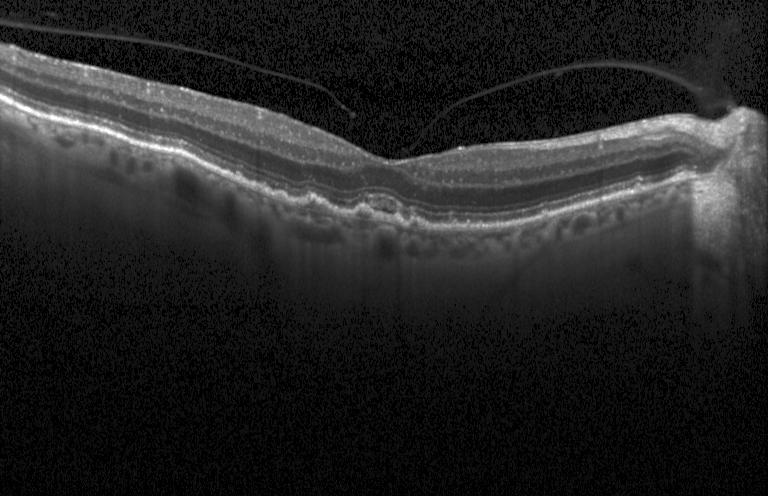
Spectral-domain optical coherence tomography. Instrument: Heidelberg Spectralis. Optical coherence tomography B-scan.
Assessment: CNV.